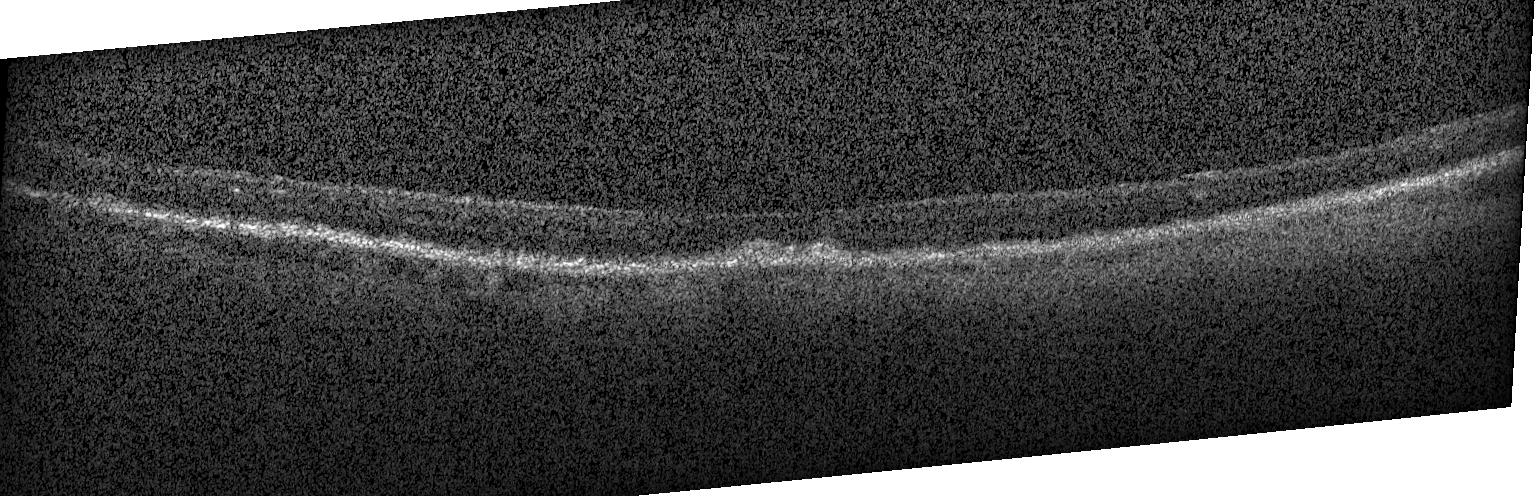

Optical coherence tomography B-scan. Heidelberg Spectralis OCT system. OCT finding: CNV.